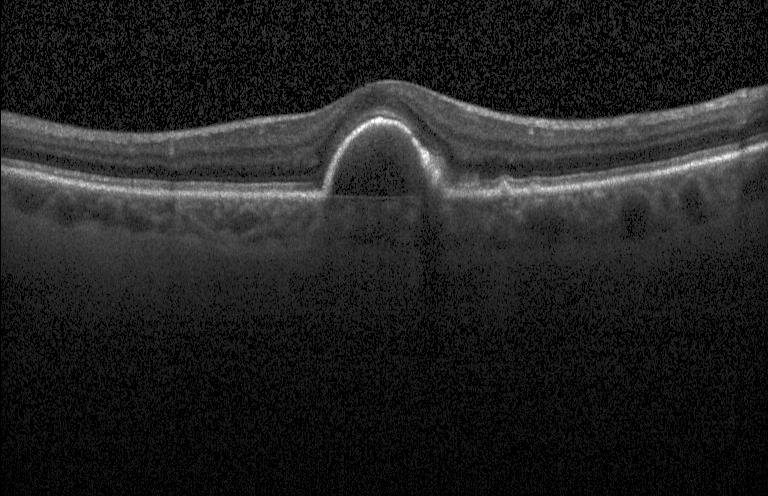

Fovea-centered · OCT line scan · acquired on a Heidelberg Spectralis — A choroidal neovascular membrane.